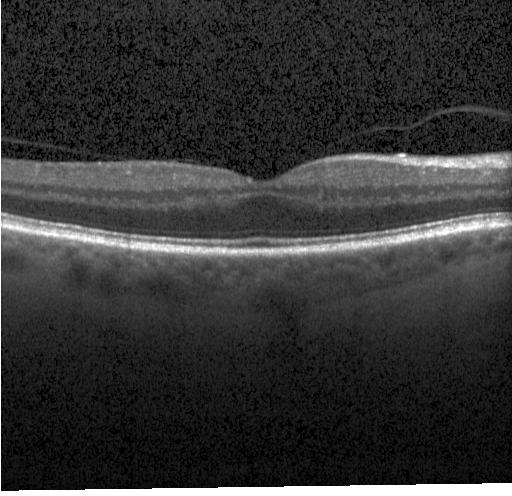 Macular OCT demonstrating neither choroidal neovascularization, diabetic macular edema, nor drusen.